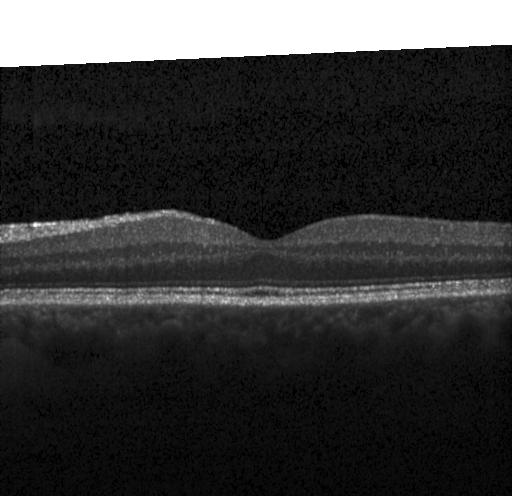 Finding: no evidence of choroidal neovascularization, diabetic macular edema, or drusen.